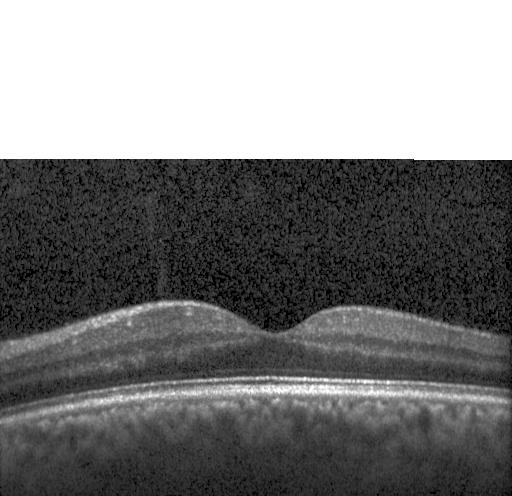 Optical coherence tomography scan. Spectral-domain optical coherence tomography. Heidelberg Spectralis OCT system. Horizontal scan through the fovea
Macular OCT: neither choroidal neovascularization, diabetic macular edema, nor drusen.